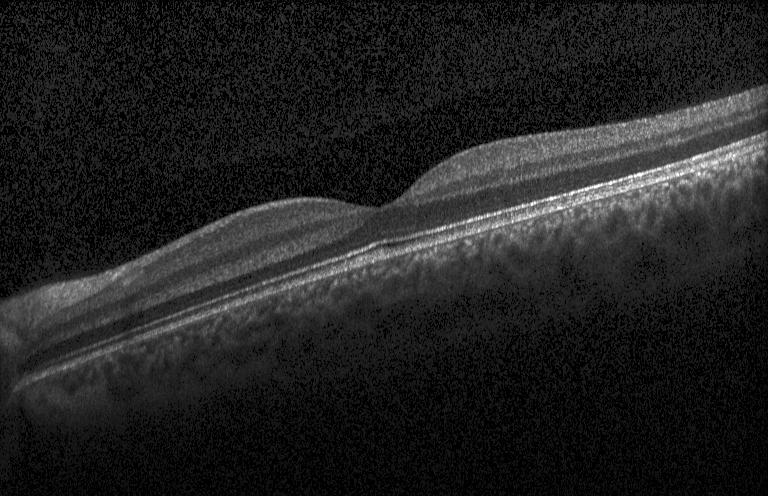 Macular scan · acquired on a Heidelberg Spectralis · SD-OCT · retinal OCT B-scan.
Impression: no choroidal neovascularization, no diabetic macular edema, and no drusen.